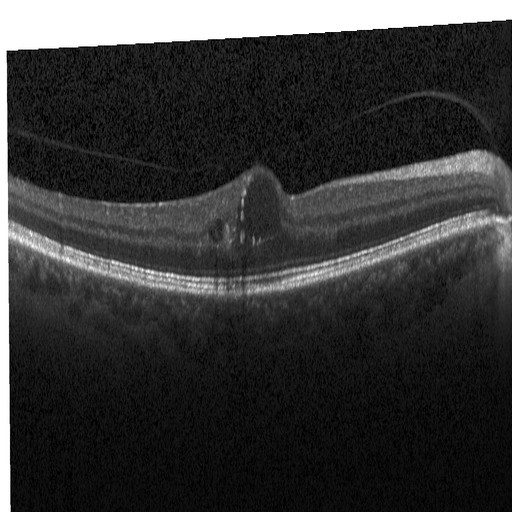

Spectral-domain OCT · OCT B-scan.
The scan shows diabetic macular edema (DME).